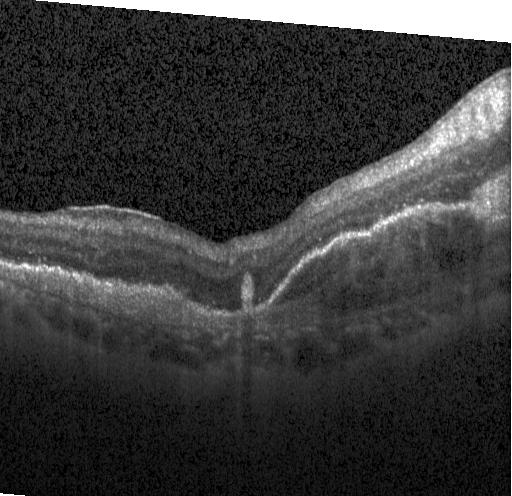
Instrument: Heidelberg Spectralis. Optical coherence tomography scan — Choroidal neovascularization.